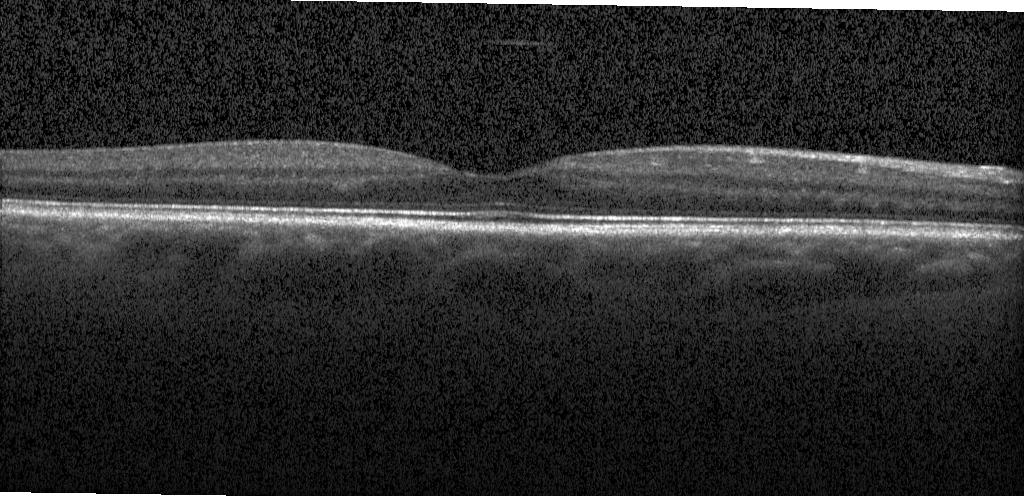
Optical coherence tomography B-scan. Diagnosis: no choroidal neovascularization, no diabetic macular edema, and no drusen.